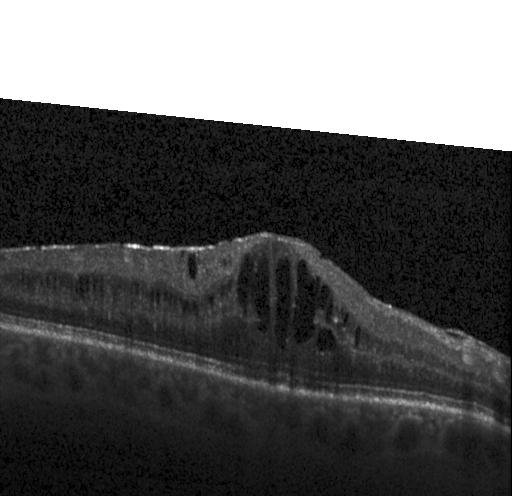
Finding: diabetic macular edema.